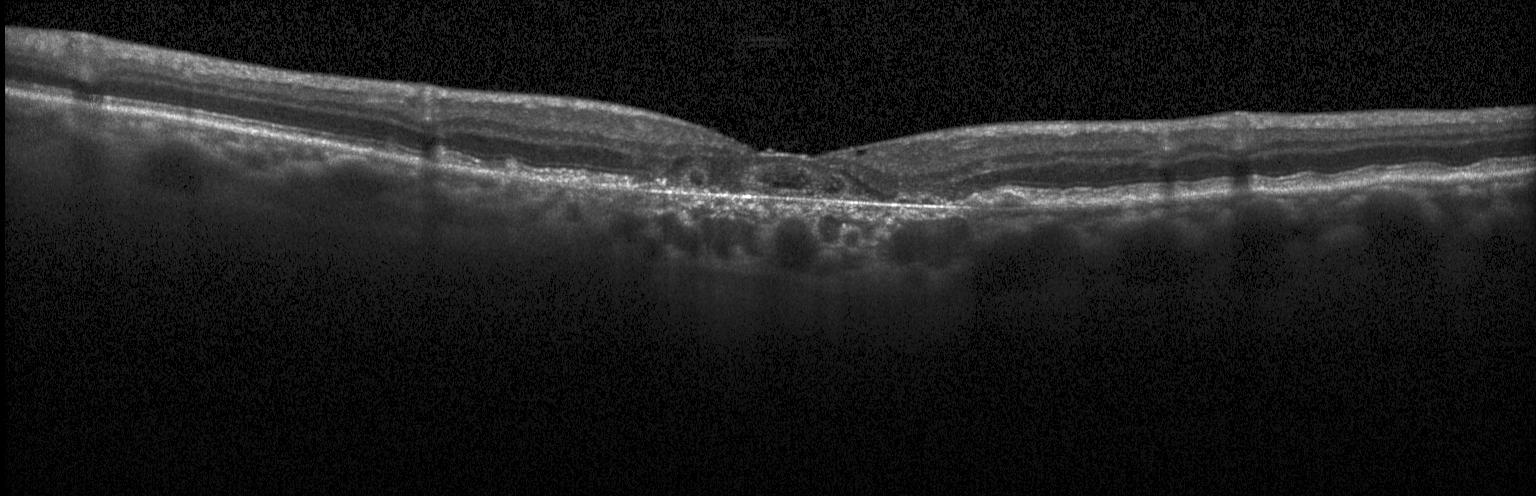 This B-scan demonstrates a choroidal neovascular membrane.